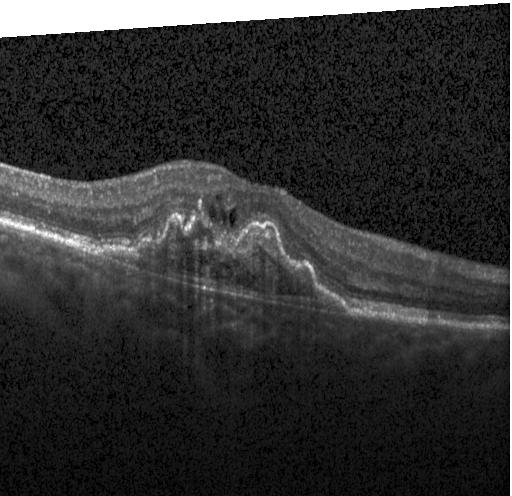

OCT finding: a choroidal neovascular membrane.